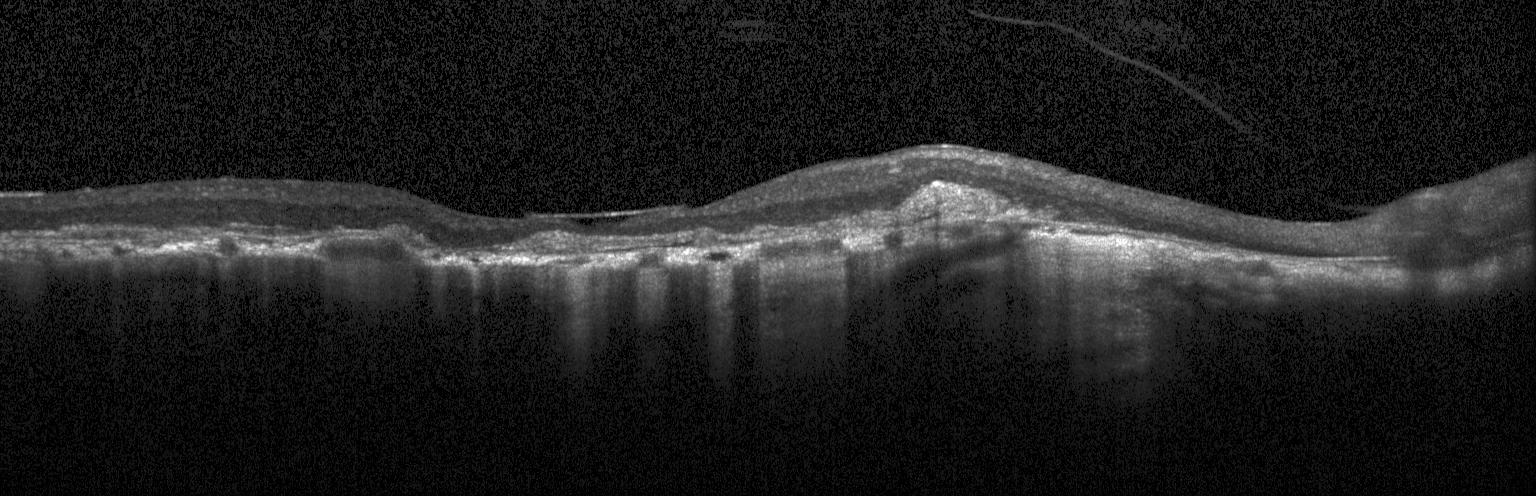 Optical coherence tomography B-scan, centered on the fovea
Diagnosis: CNV.